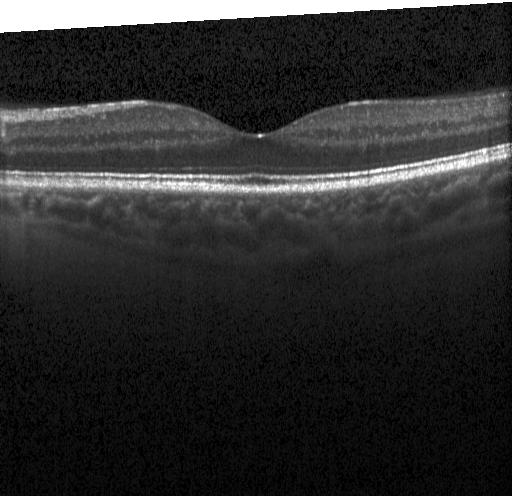 Through the macula, spectral-domain optical coherence tomography, retinal OCT cross-section, instrument: Heidelberg Spectralis
The scan shows no choroidal neovascularization, diabetic macular edema, or drusen.